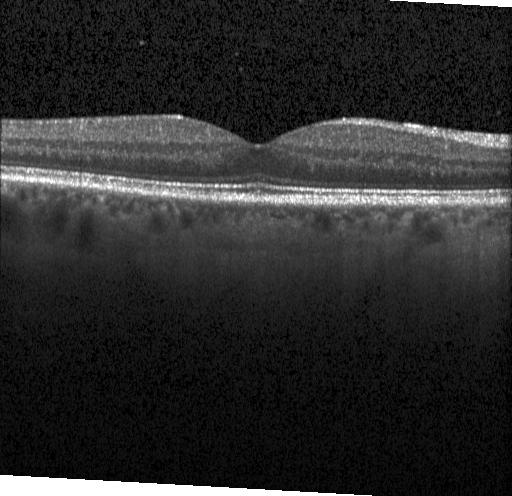

OCT line scan
Assessment: neither CNV, DME, nor drusen.